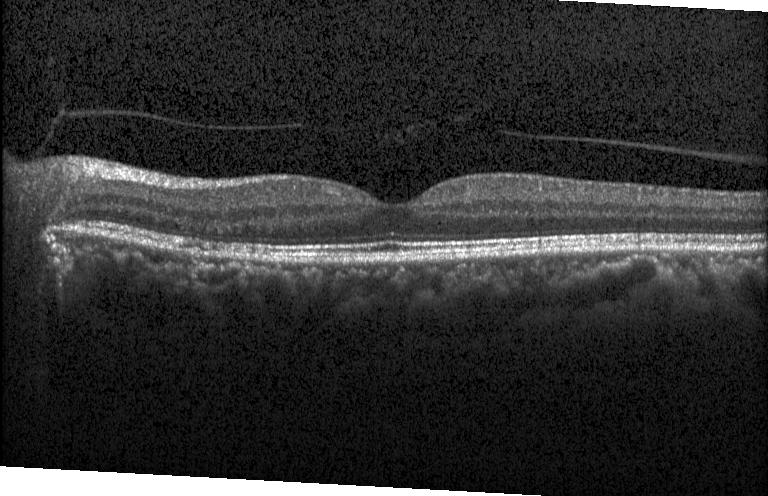 Dx: neither choroidal neovascularization, diabetic macular edema, nor drusen.